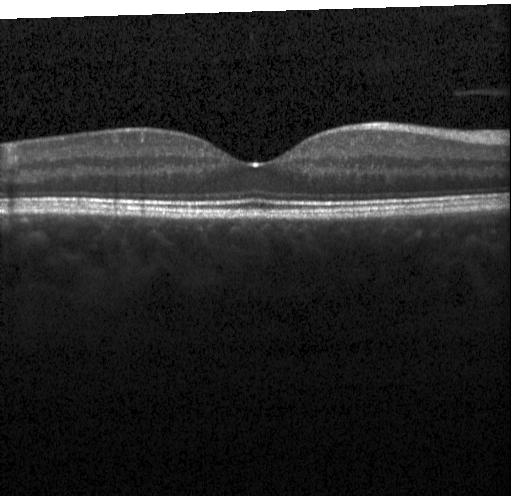

OCT finding: no choroidal neovascularization, diabetic macular edema, or drusen.